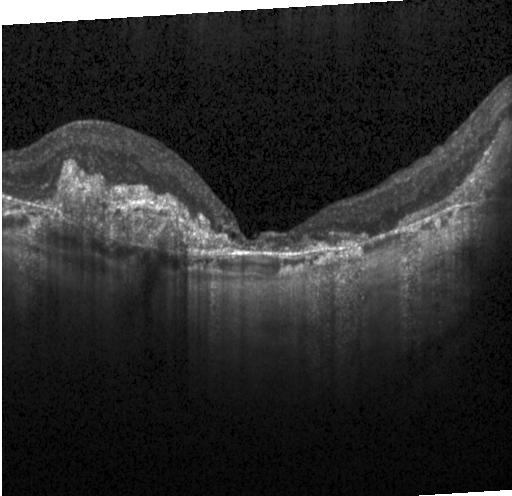
Heidelberg Spectralis OCT system; horizontal scan through the fovea; optical coherence tomography B-scan — Macular OCT: a choroidal neovascular membrane.